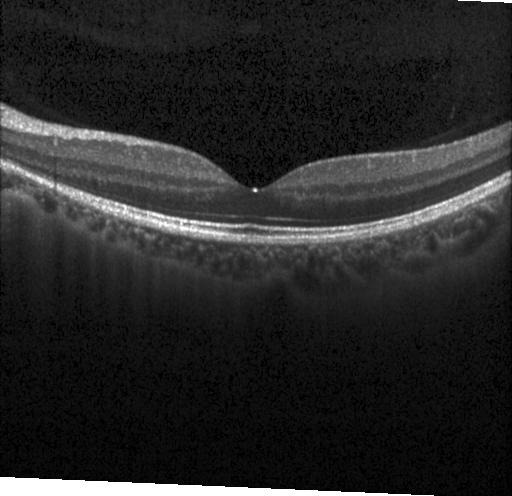
Diagnosis: no evidence of CNV, DME, or drusen.